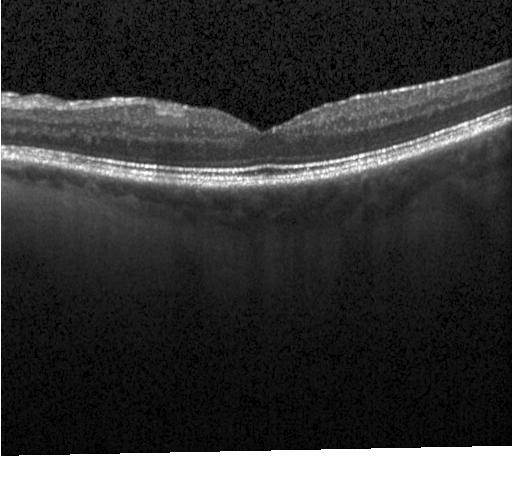 Retinal OCT cross-section showing no choroidal neovascularization, no diabetic macular edema, and no drusen.